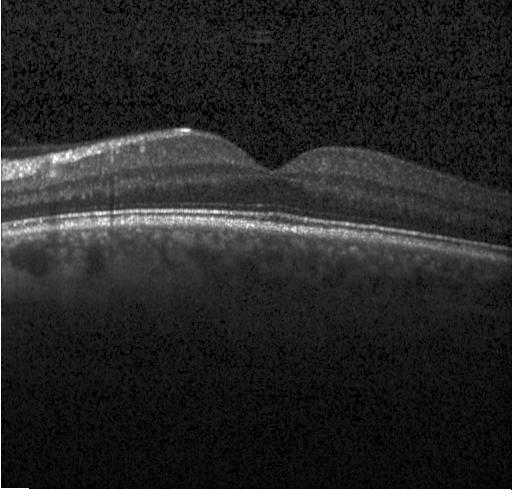
Heidelberg Spectralis, retinal OCT cross-section, spectral-domain optical coherence tomography
Finding: no choroidal neovascularization, no diabetic macular edema, and no drusen.